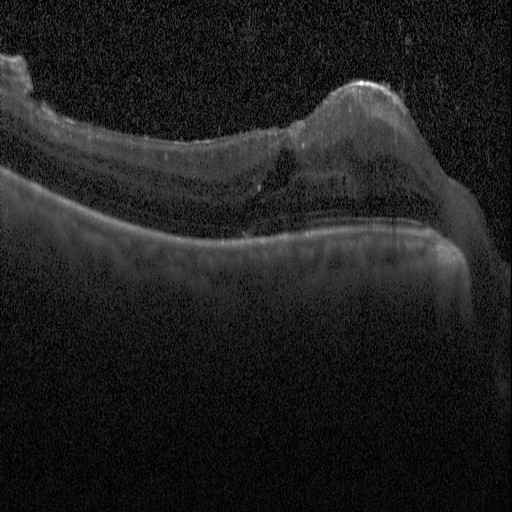

Impression: DME.